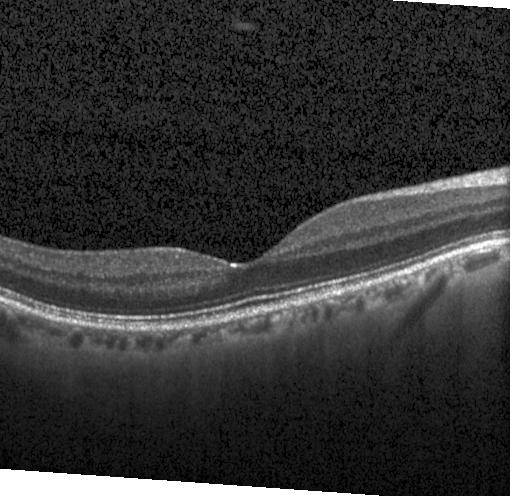 Acquired on a Heidelberg Spectralis; optical coherence tomography scan — The scan shows no choroidal neovascularization, diabetic macular edema, or drusen.